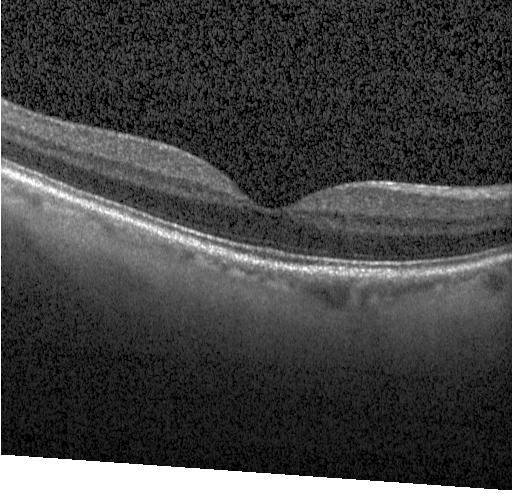
OCT finding: no choroidal neovascularization, no diabetic macular edema, and no drusen.